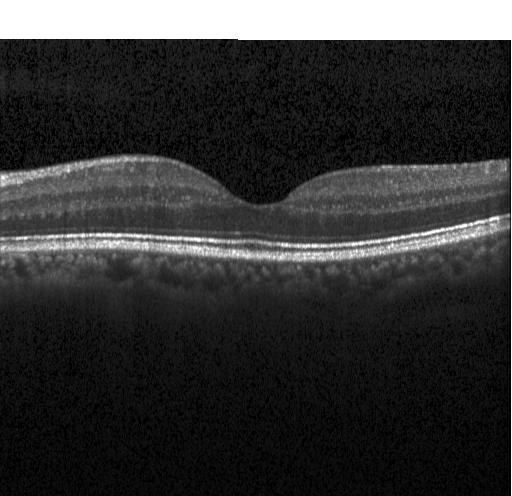

Finding: no evidence of CNV, DME, or drusen.